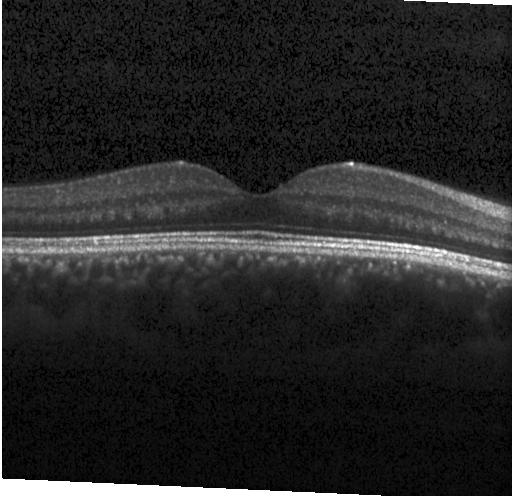
Retinal OCT cross-section — Diagnosis: neither choroidal neovascularization, diabetic macular edema, nor drusen.